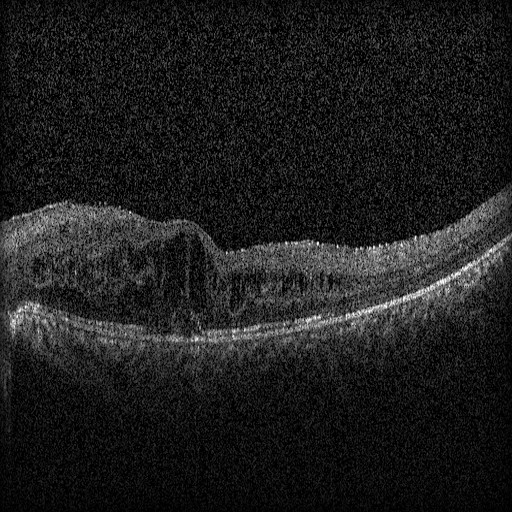
Retinal OCT cross-section showing DME.